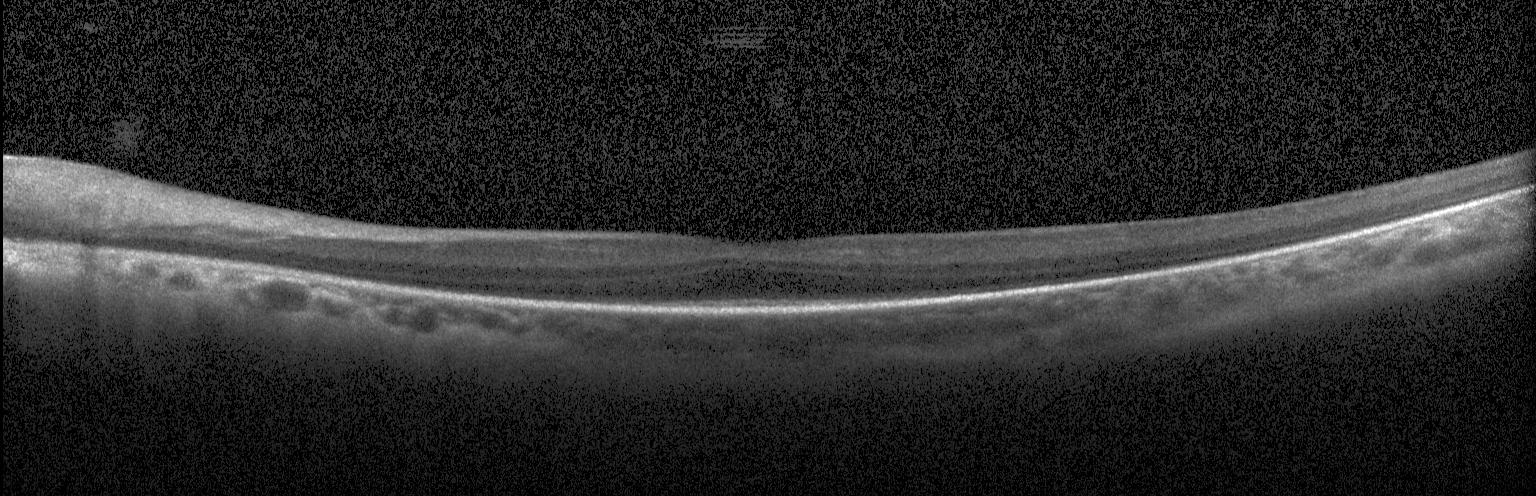
Retinal OCT B-scan, fovea-centered, SD-OCT.
Dx: no evidence of choroidal neovascularization, diabetic macular edema, or drusen.